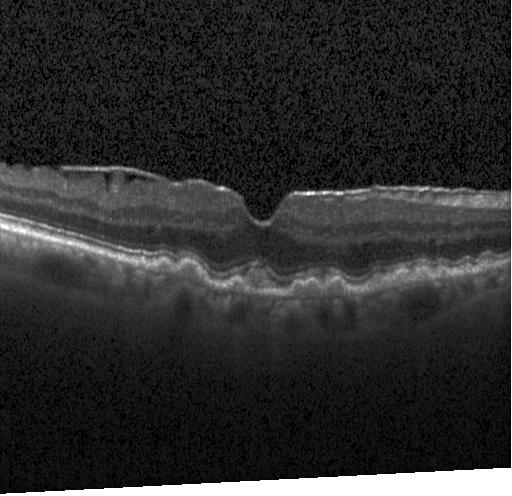 Fovea-centered, retinal OCT cross-section. Dx: sub-RPE drusenoid deposits.